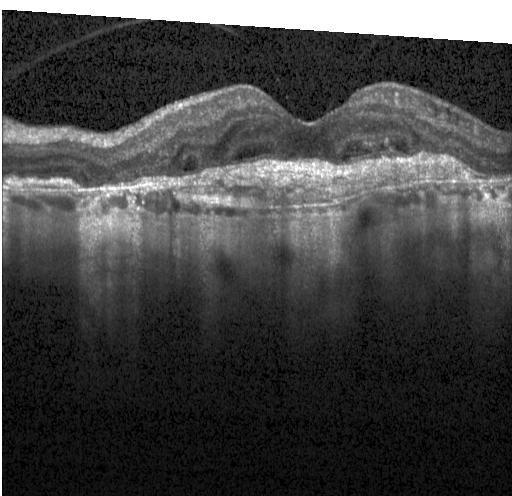

Retinal OCT B-scan
Assessment: a choroidal neovascular membrane.